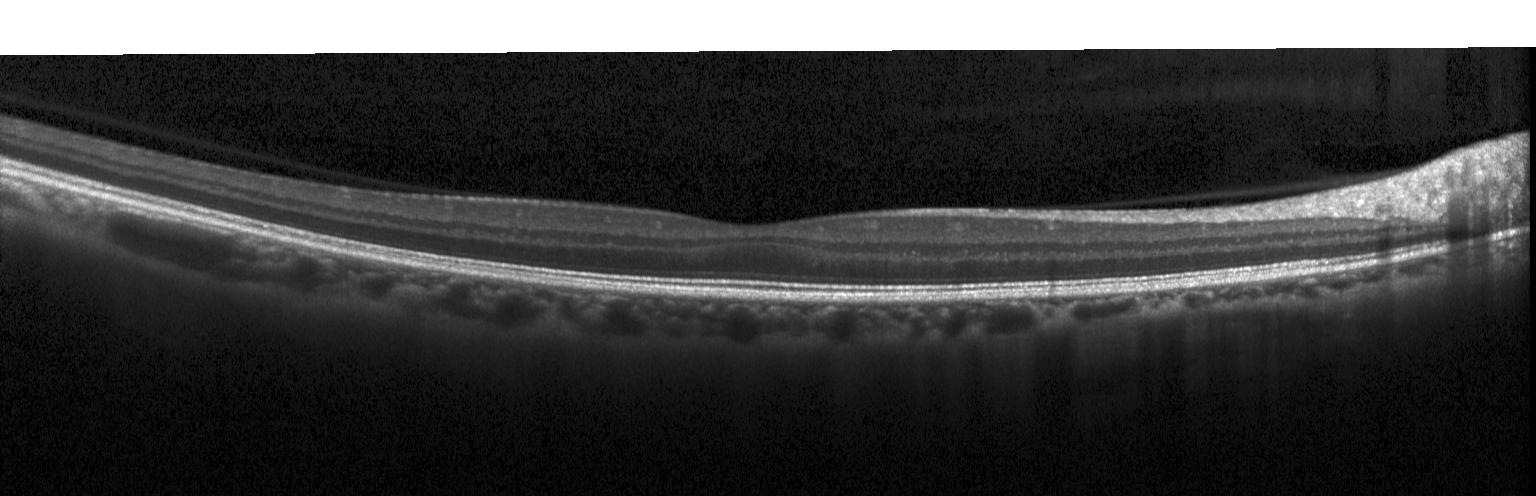 Spectral-domain optical coherence tomography; acquired on a Heidelberg Spectralis; optical coherence tomography scan. The scan shows no choroidal neovascularization, no diabetic macular edema, and no drusen.